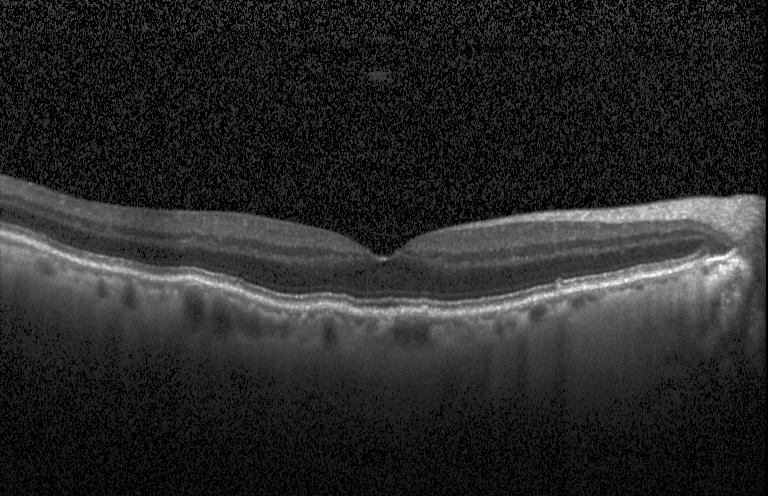 Drusen.